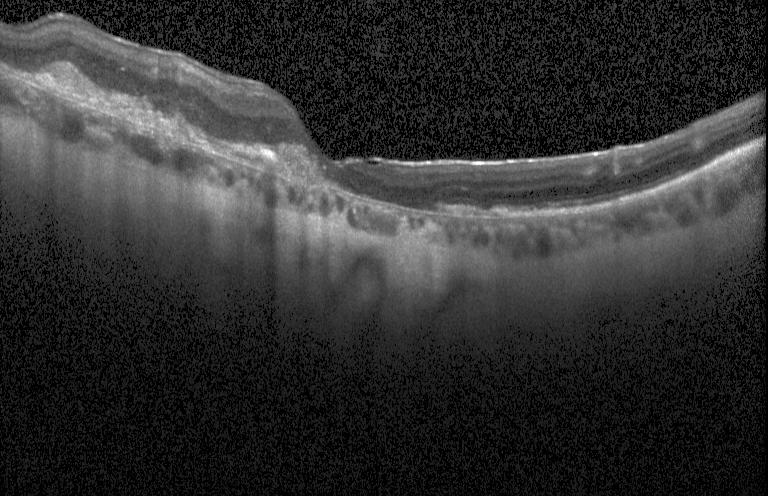
Macular OCT: a choroidal neovascular membrane.